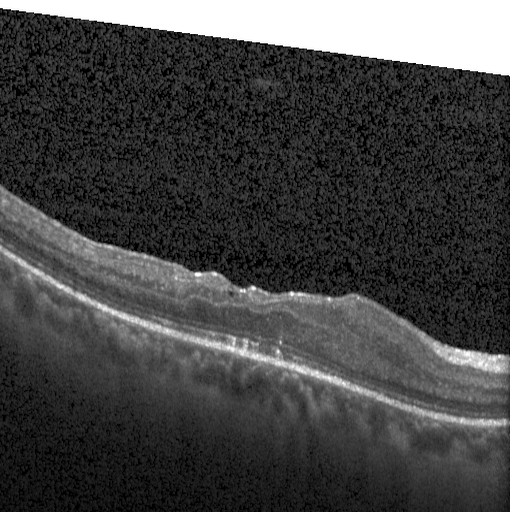
Macular OCT: DME.